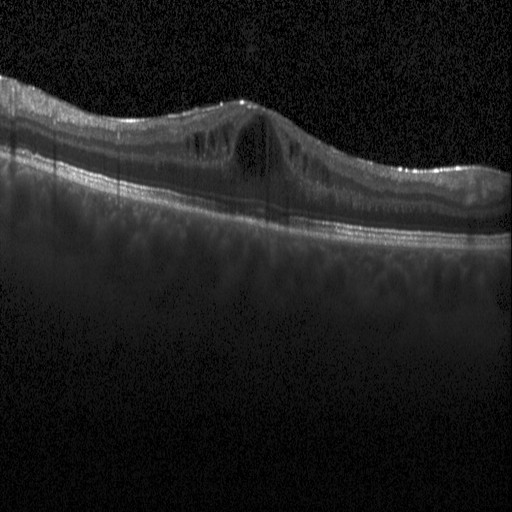 Retinal OCT cross-section · spectral-domain optical coherence tomography. Finding: DME.